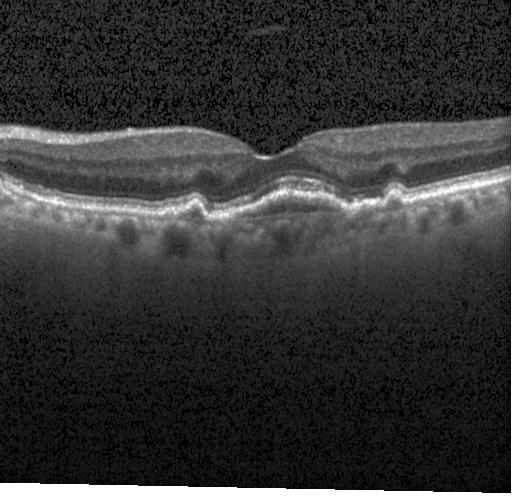

Heidelberg Spectralis OCT system · retinal OCT cross-section · spectral-domain OCT
Diagnosis: a choroidal neovascular membrane.